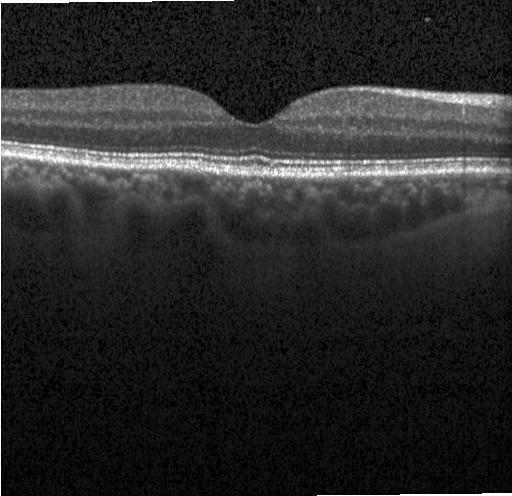

Retinal OCT cross-section; SD-OCT
Diagnosis: no choroidal neovascularization, no diabetic macular edema, and no drusen.